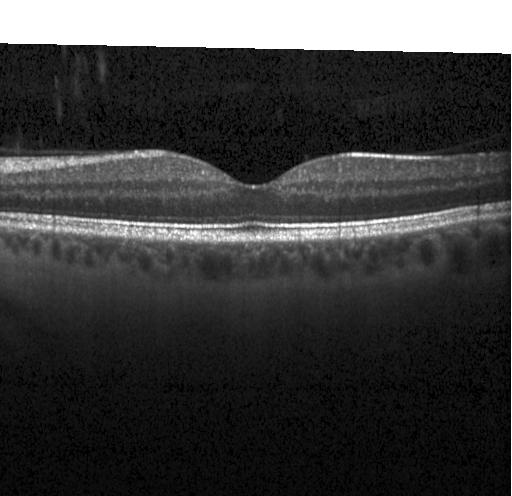

The scan shows no CNV, no DME, and no drusen.